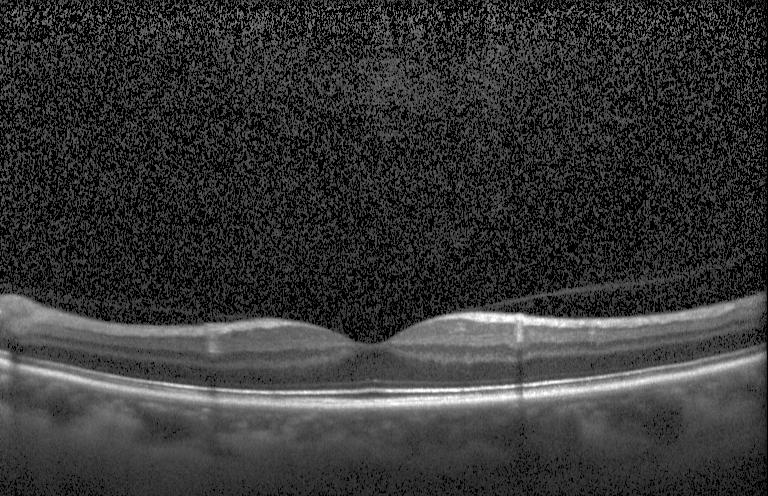
Retinal OCT cross-section, through the macula
This B-scan demonstrates no CNV, DME, or drusen.